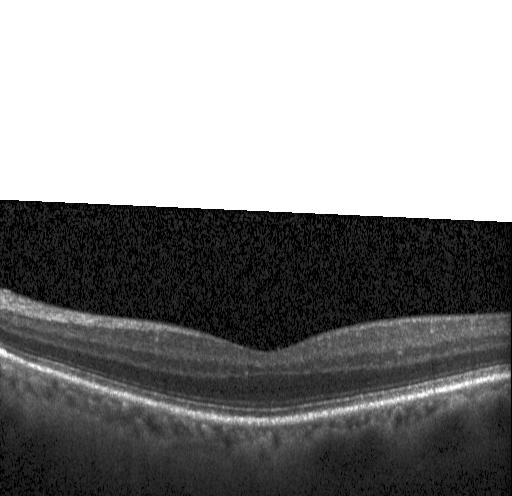
Macular OCT demonstrating neither choroidal neovascularization, diabetic macular edema, nor drusen.